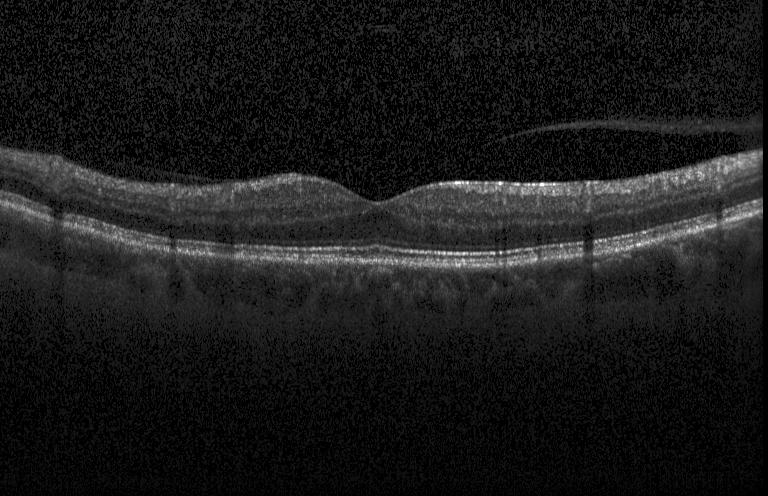 Through the macula. Heidelberg Spectralis OCT system. Spectral-domain optical coherence tomography. Optical coherence tomography B-scan.
Impression: neither CNV, DME, nor drusen.